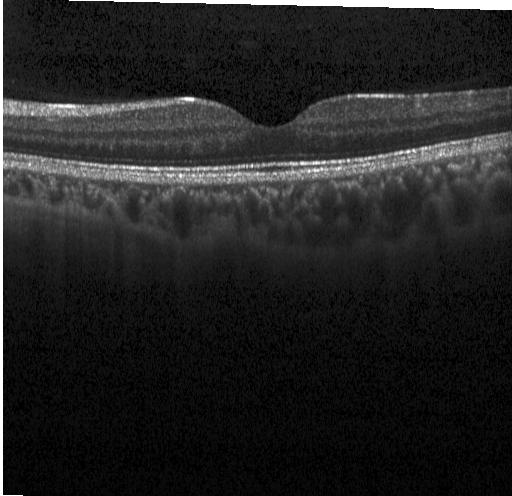
OCT line scan. Heidelberg Spectralis. Spectral-domain OCT. This B-scan demonstrates no CNV, DME, or drusen.